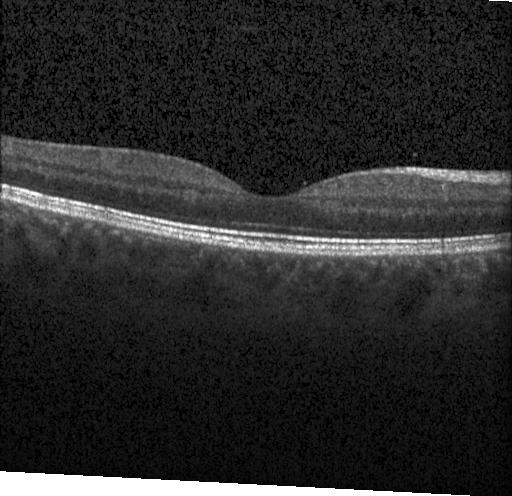
This B-scan demonstrates no CNV, DME, or drusen.